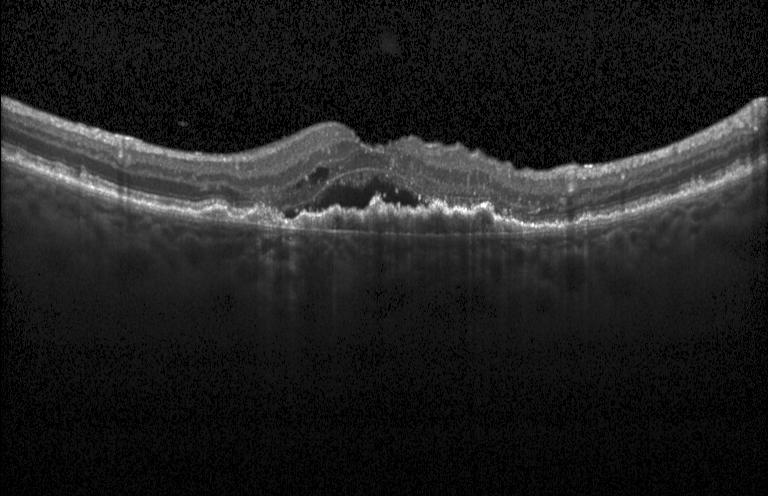

Centered on the fovea · acquired on a Heidelberg Spectralis · SD-OCT · optical coherence tomography B-scan. Choroidal neovascularization.